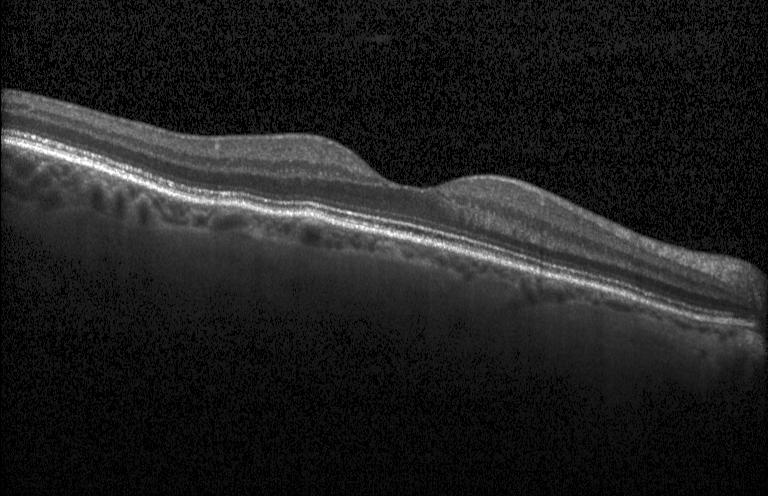

Fovea-centered. Optical coherence tomography B-scan. Impression: no choroidal neovascularization, diabetic macular edema, or drusen.